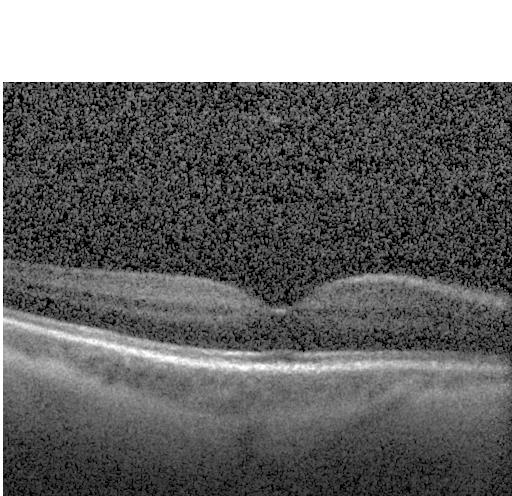 OCT line scan. Heidelberg Spectralis. The scan shows no choroidal neovascularization, diabetic macular edema, or drusen.